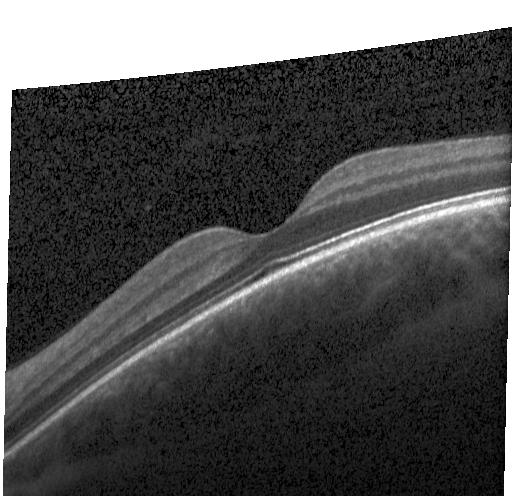 Assessment: no choroidal neovascularization, diabetic macular edema, or drusen.